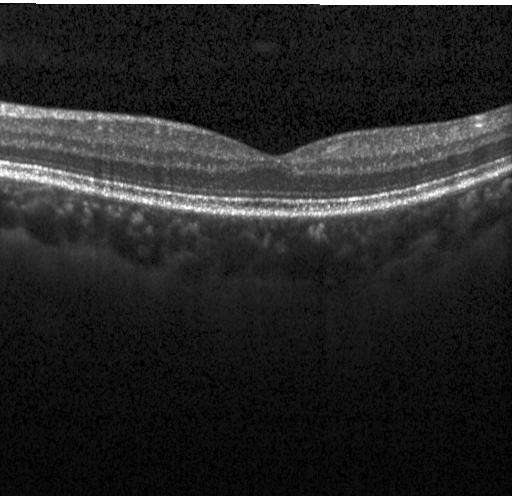

Macular OCT: no choroidal neovascularization, diabetic macular edema, or drusen.